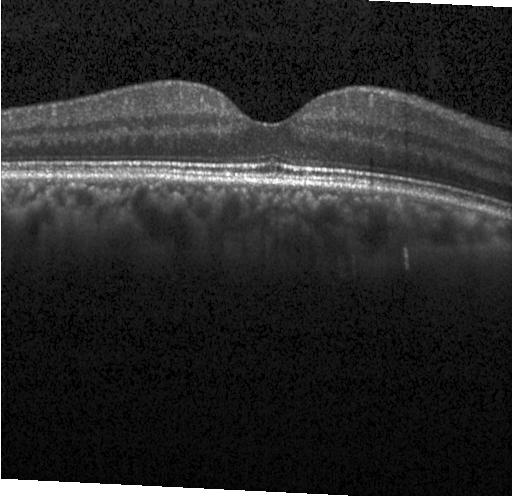
Retinal OCT cross-section showing no evidence of choroidal neovascularization, diabetic macular edema, or drusen.